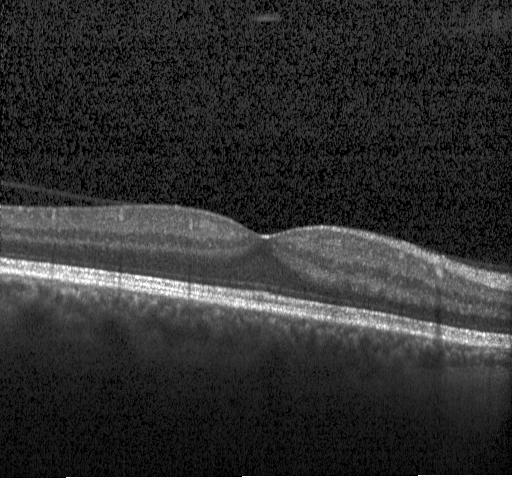
Impression: no CNV, no DME, and no drusen.